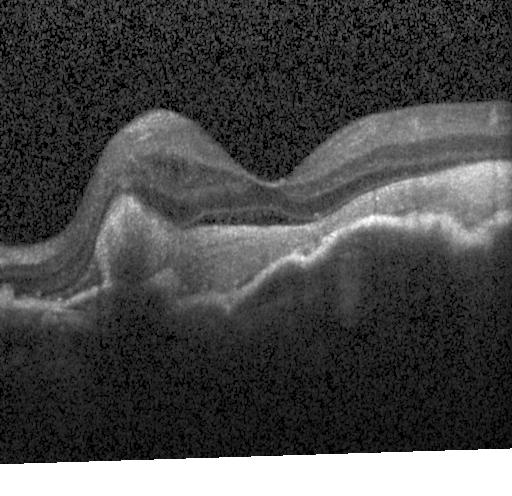 Optical coherence tomography B-scan, spectral-domain OCT
Macular OCT: a choroidal neovascular membrane.